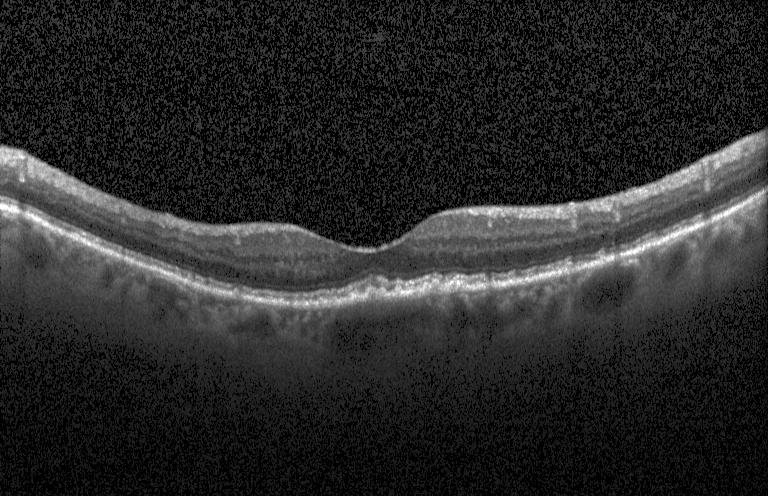 Retinal OCT B-scan, acquired on a Heidelberg Spectralis
Diagnosis: drusen.